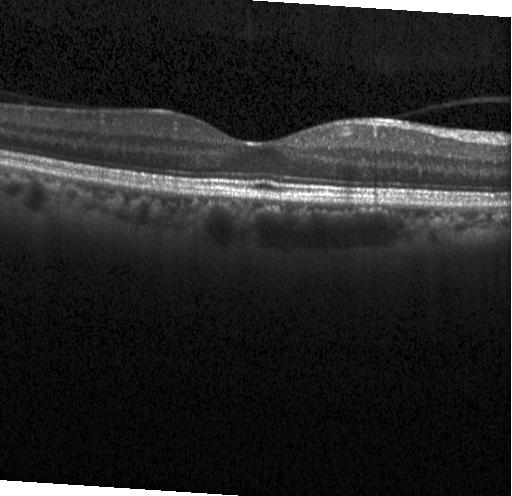

The scan shows no choroidal neovascularization, diabetic macular edema, or drusen.